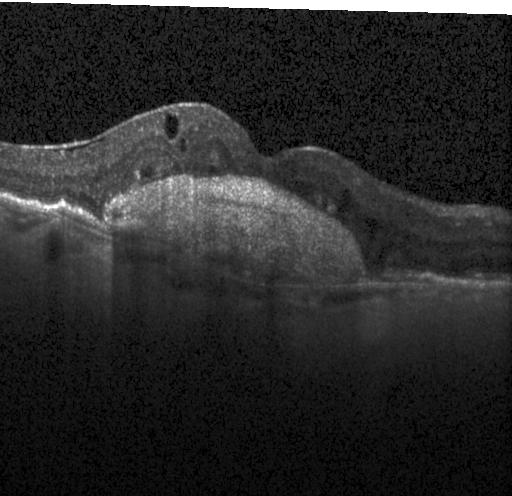

Heidelberg Spectralis OCT system; optical coherence tomography B-scan.
Finding: choroidal neovascularization (CNV).